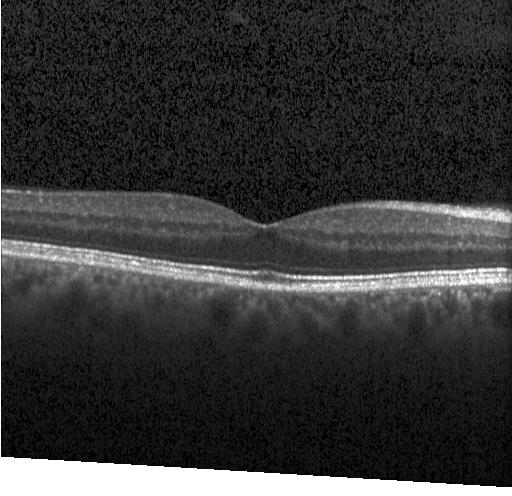
Impression: no evidence of CNV, DME, or drusen.